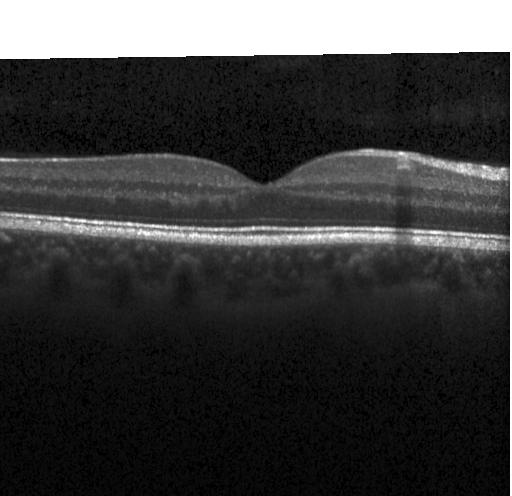

Spectral-domain optical coherence tomography; optical coherence tomography B-scan; centered on the fovea
Assessment: neither CNV, DME, nor drusen.